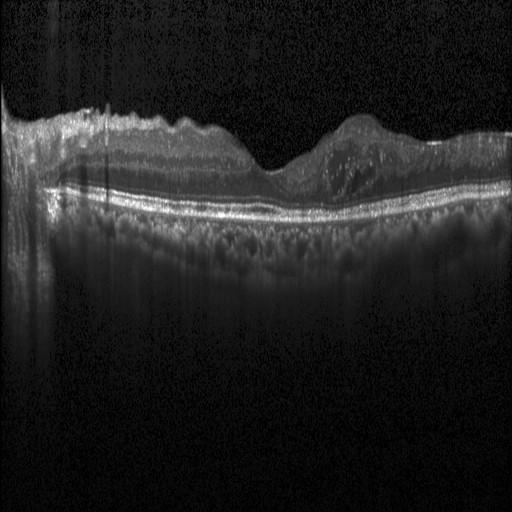

Horizontal scan through the fovea · optical coherence tomography scan · spectral-domain OCT
Finding: DME.